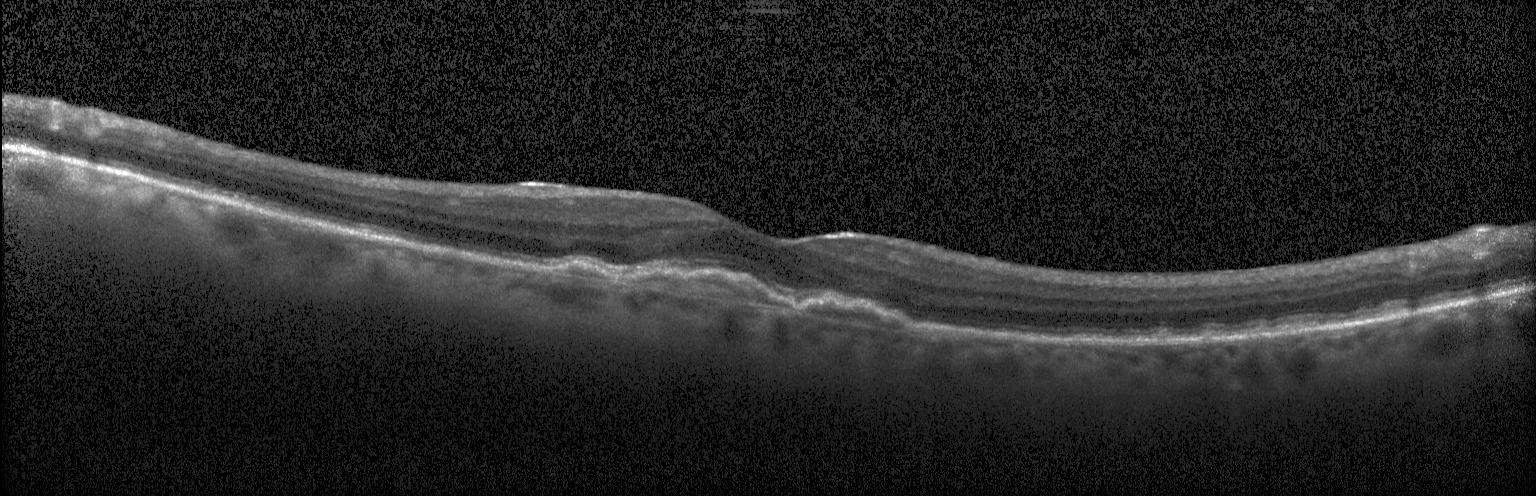

This B-scan demonstrates a choroidal neovascular membrane.